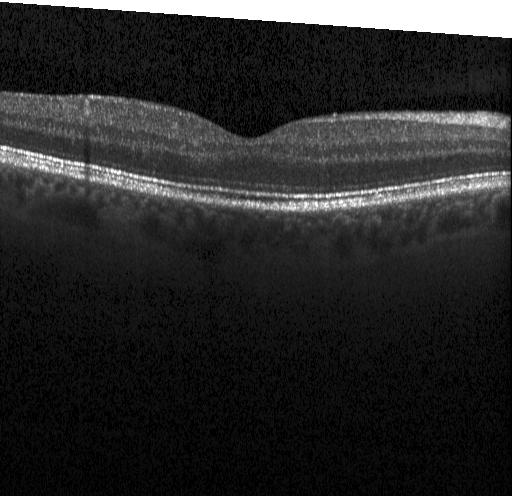 OCT finding: no CNV, DME, or drusen.